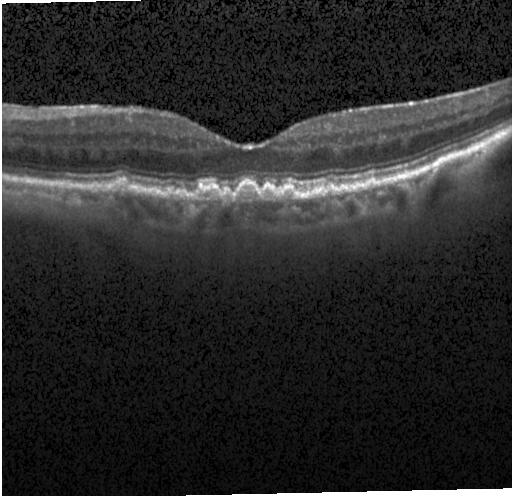

OCT scan showing sub-RPE drusenoid deposits.